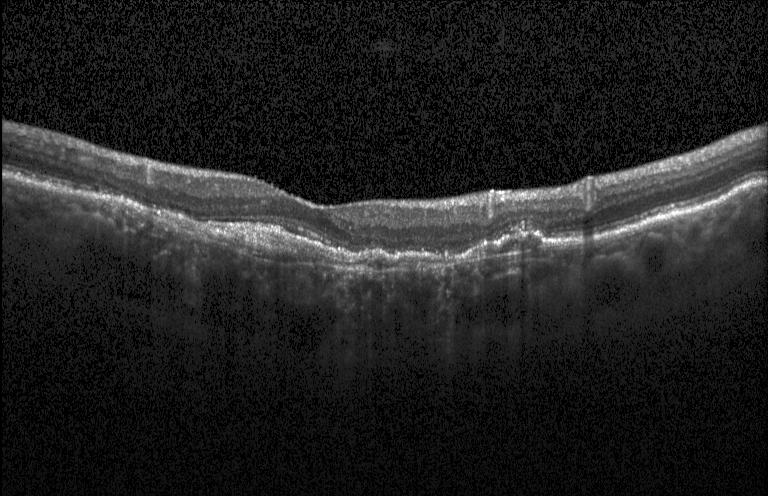
Spectral-domain optical coherence tomography · horizontal scan through the fovea · Heidelberg Spectralis OCT system · OCT B-scan — Assessment: choroidal neovascularization.